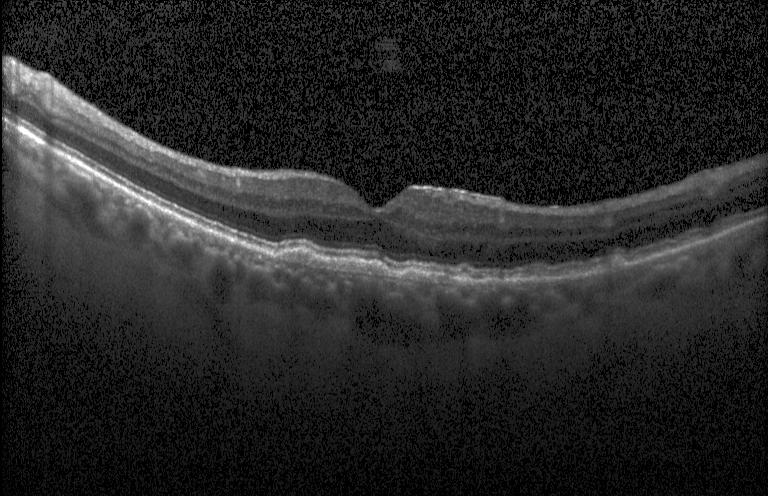
Impression: CNV.